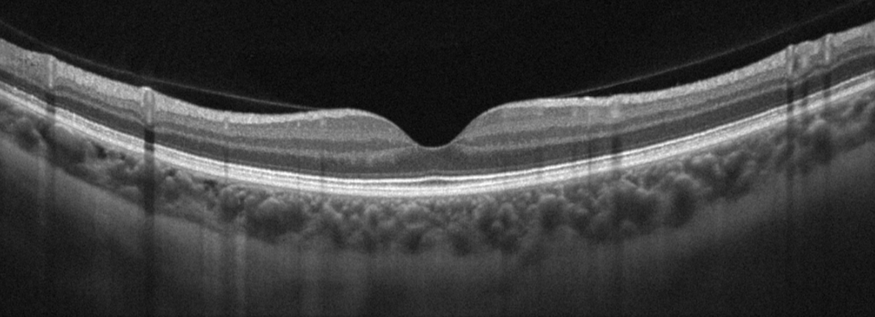 Fovea-centered; optical coherence tomography scan.
No AMD, DME, ERM, RAO, RVO, or VID.